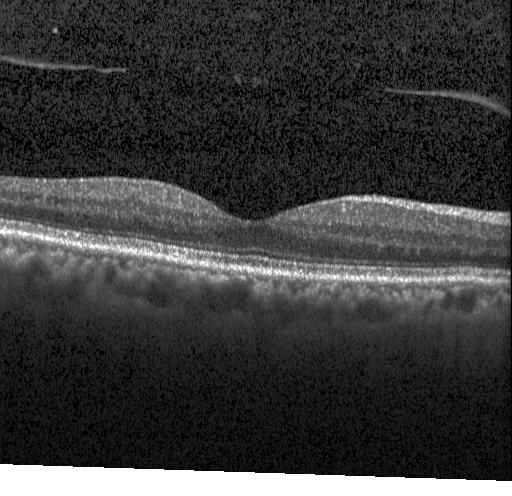
OCT B-scan.
Impression: no choroidal neovascularization, diabetic macular edema, or drusen.